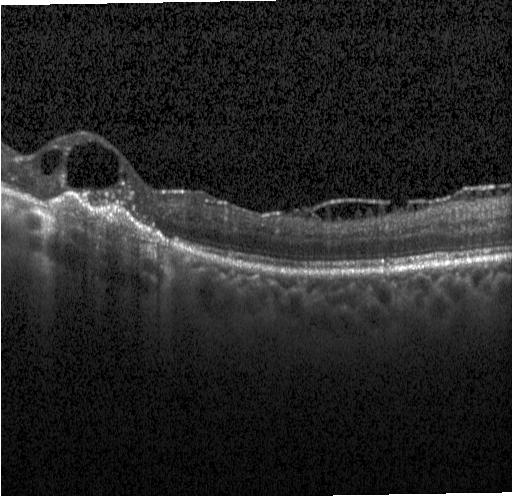
Spectral-domain optical coherence tomography, retinal OCT B-scan, instrument: Heidelberg Spectralis, macular scan
Diagnosis: a choroidal neovascular membrane.